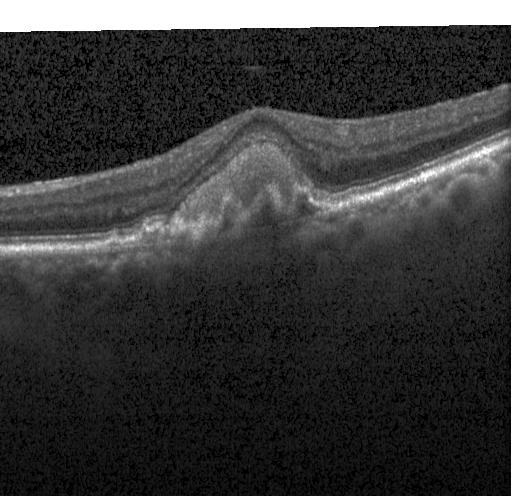
OCT B-scan showing CNV.